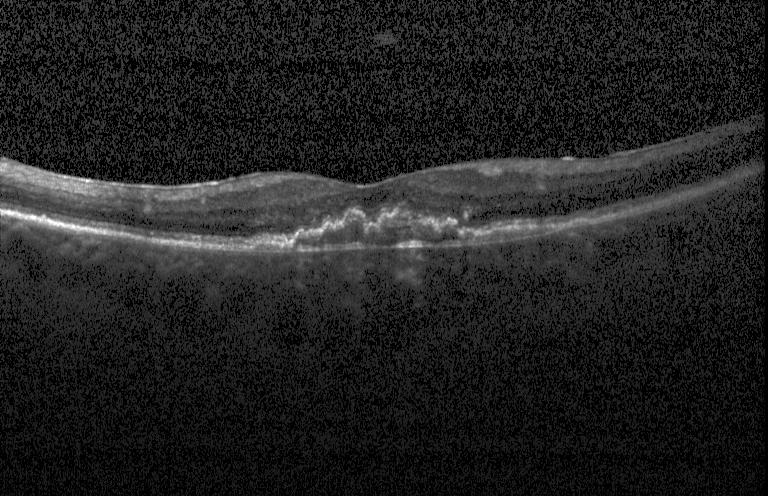
OCT line scan. Finding: CNV.